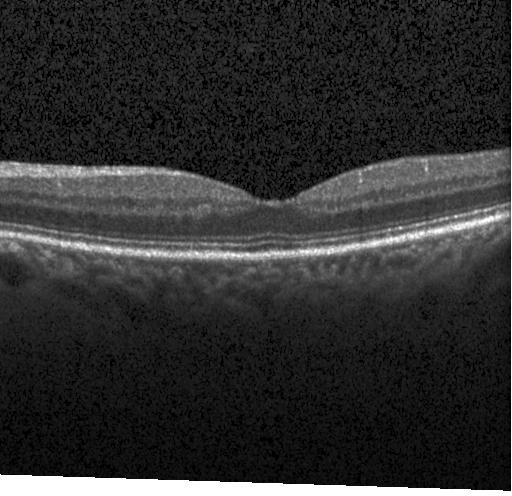 Retinal OCT B-scan, acquired on a Heidelberg Spectralis, spectral-domain OCT — Finding: neither CNV, DME, nor drusen.